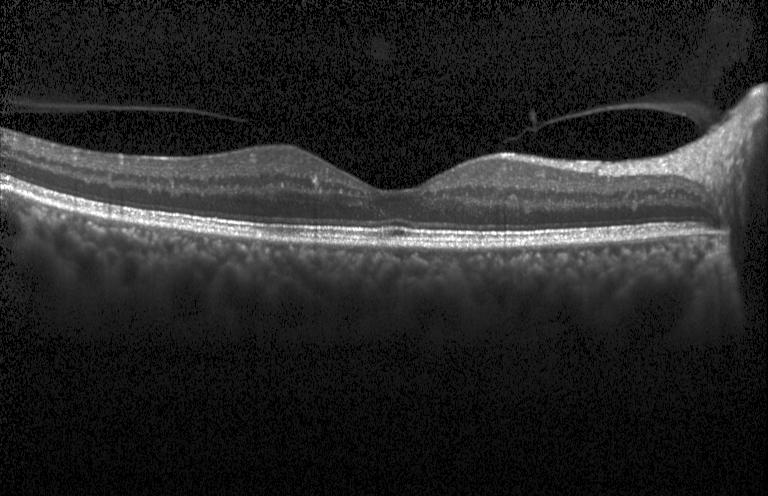

OCT B-scan
Diagnosis: no evidence of CNV, DME, or drusen.